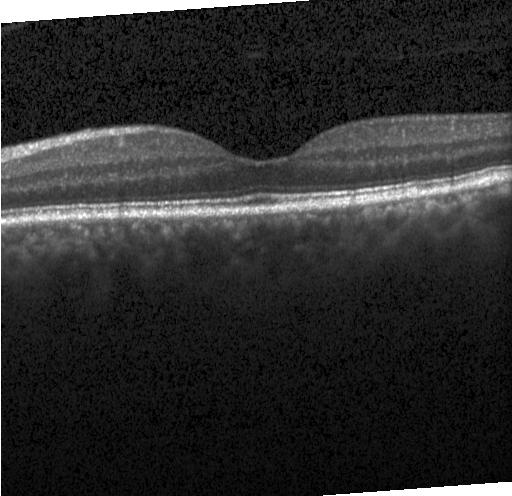

Spectral-domain OCT, through the macula, instrument: Heidelberg Spectralis, retinal OCT cross-section.
OCT finding: no evidence of choroidal neovascularization, diabetic macular edema, or drusen.